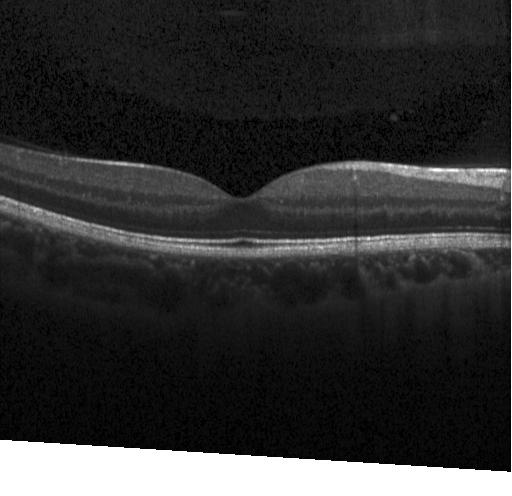
Diagnosis: neither choroidal neovascularization, diabetic macular edema, nor drusen.